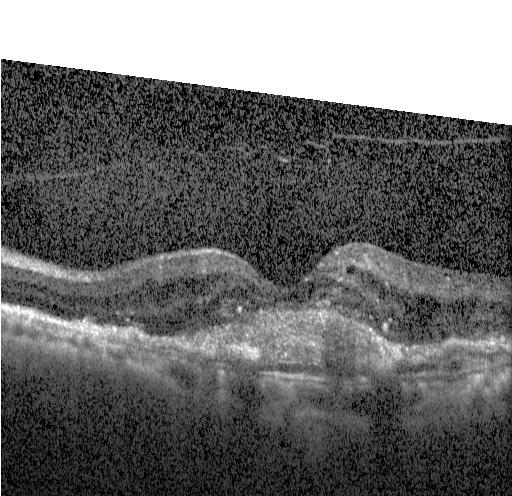

Retinal OCT B-scan. Finding: choroidal neovascularization (CNV).